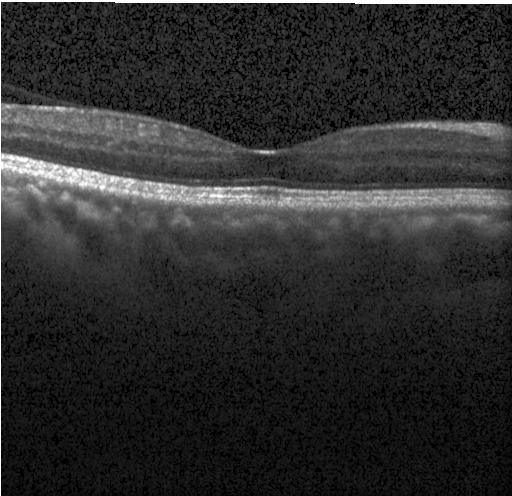 OCT B-scan showing neither CNV, DME, nor drusen.